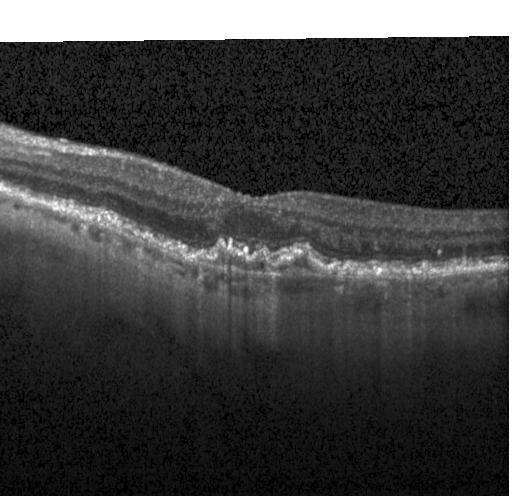

OCT B-scan.
Macular OCT: choroidal neovascularization (CNV).